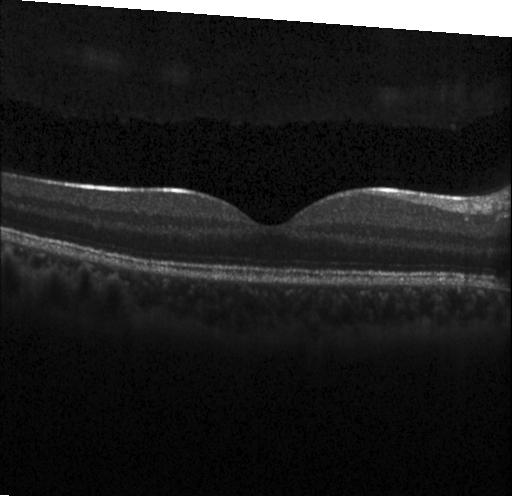

Heidelberg Spectralis OCT system, spectral-domain OCT, retinal OCT cross-section — Impression: no choroidal neovascularization, no diabetic macular edema, and no drusen.